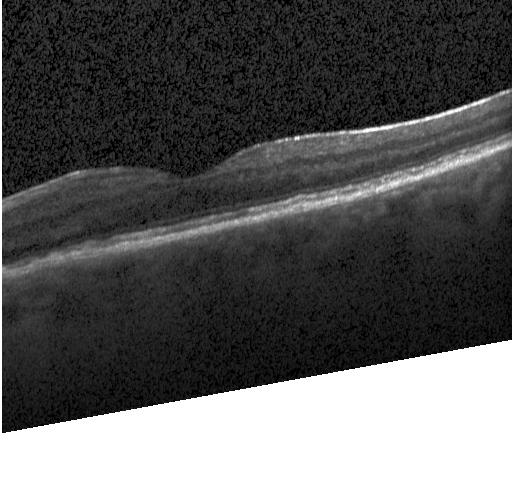
Optical coherence tomography B-scan · through the macula · spectral-domain OCT · instrument: Heidelberg Spectralis — Finding: no choroidal neovascularization, diabetic macular edema, or drusen.